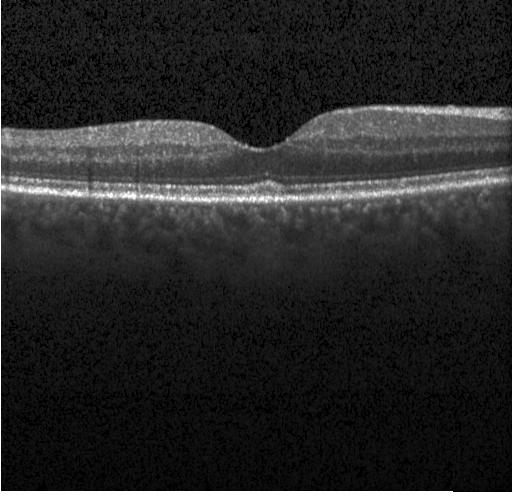 Horizontal scan through the fovea. OCT B-scan.
Macular OCT: no evidence of choroidal neovascularization, diabetic macular edema, or drusen.